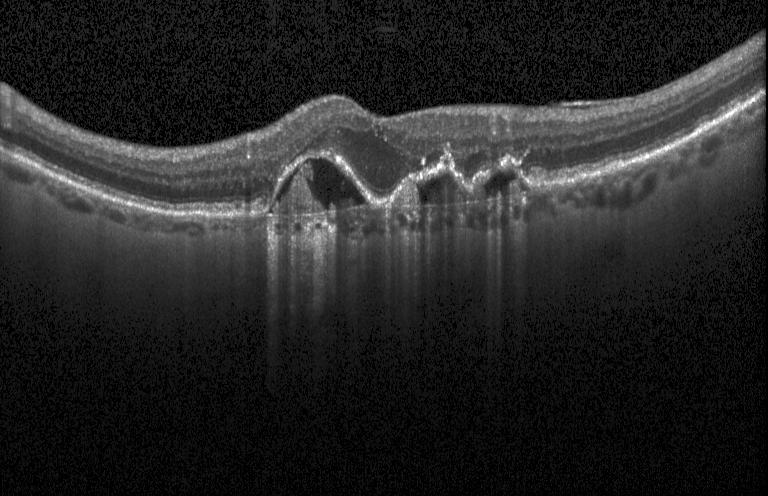
Optical coherence tomography B-scan, through the macula. Finding: choroidal neovascularization (CNV).